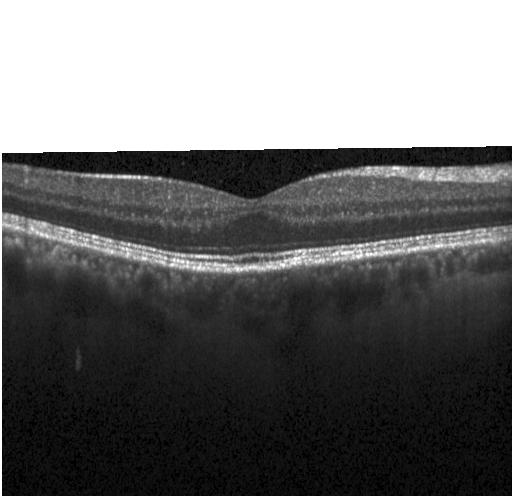

Heidelberg Spectralis · optical coherence tomography scan · through the macula · spectral-domain OCT. The scan shows no choroidal neovascularization, no diabetic macular edema, and no drusen.